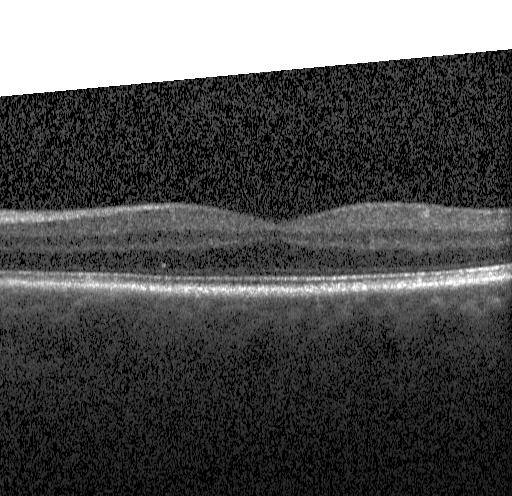 Retinal OCT B-scan
The scan shows neither choroidal neovascularization, diabetic macular edema, nor drusen.